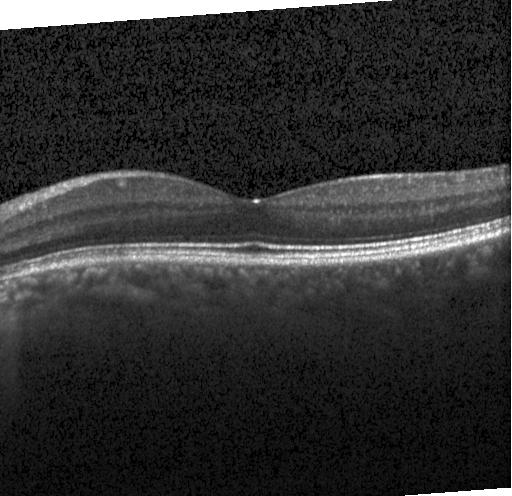 Optical coherence tomography scan — Diagnosis: no CNV, no DME, and no drusen.